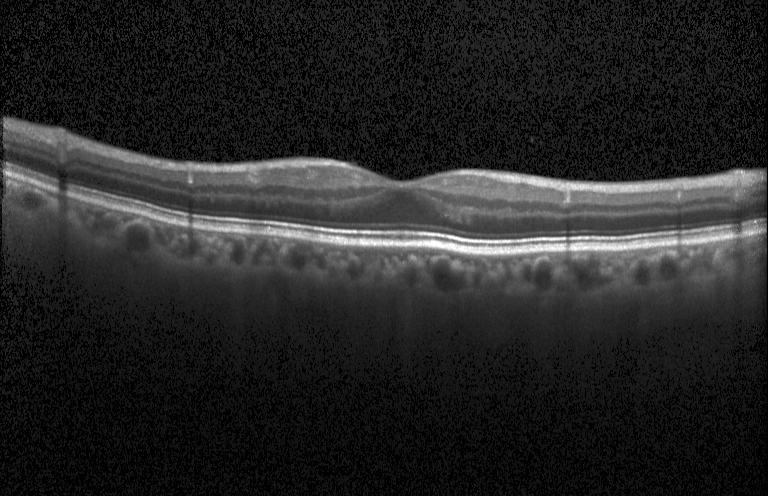 Optical coherence tomography scan; macular scan
Impression: no choroidal neovascularization, diabetic macular edema, or drusen.